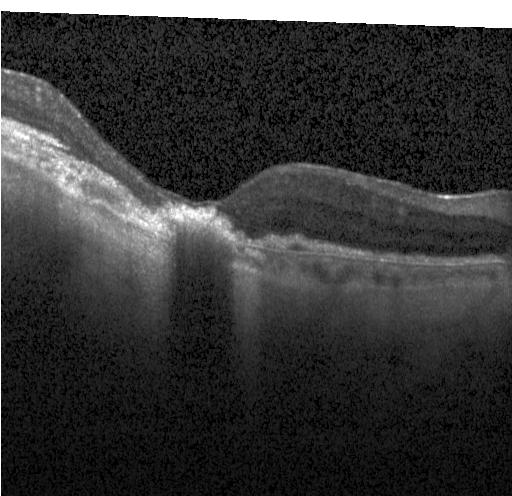

The scan shows choroidal neovascularization.